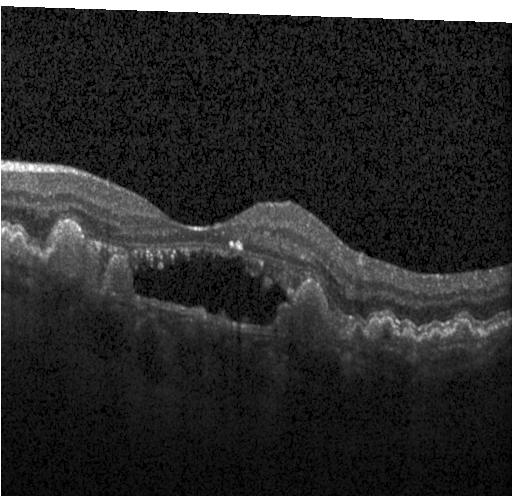

Retinal OCT B-scan. Finding: a choroidal neovascular membrane.